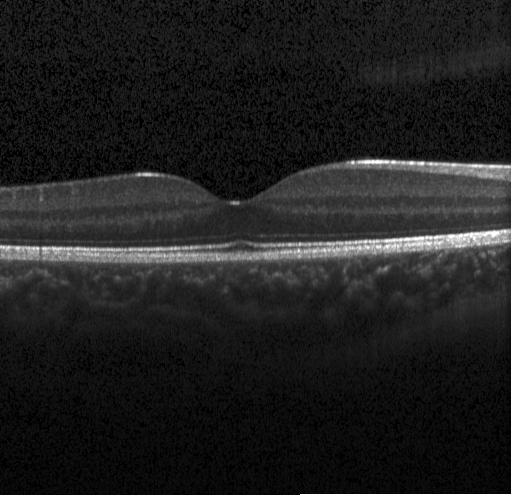
Retinal OCT cross-section showing no CNV, DME, or drusen.